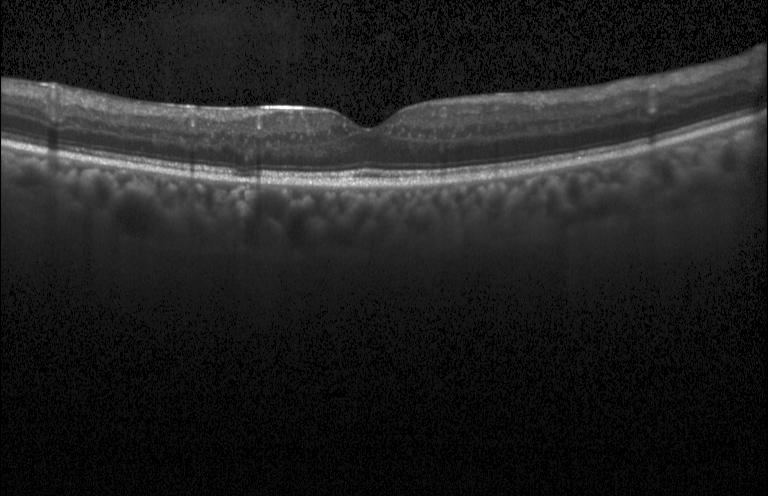

Optical coherence tomography scan; acquired on a Heidelberg Spectralis; centered on the fovea — Diagnosis: no CNV, no DME, and no drusen.